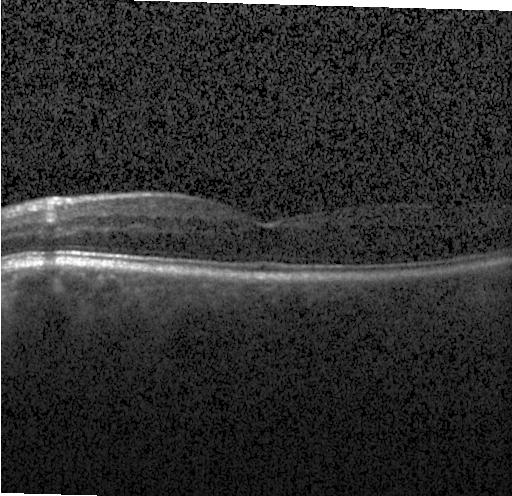

SD-OCT. Macular scan. Optical coherence tomography scan. Instrument: Heidelberg Spectralis — Diagnosis: neither choroidal neovascularization, diabetic macular edema, nor drusen.